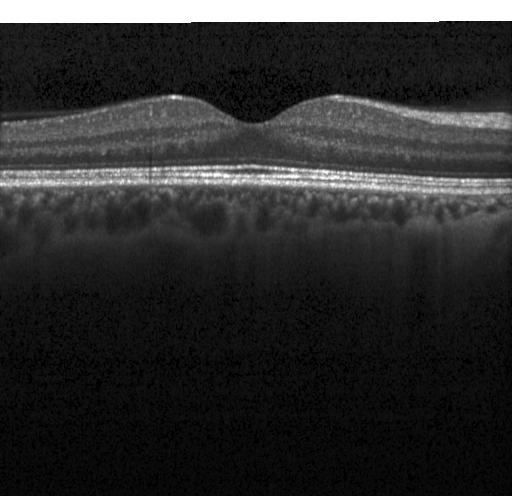

Horizontal scan through the fovea · SD-OCT · optical coherence tomography scan. Diagnosis: no choroidal neovascularization, no diabetic macular edema, and no drusen.